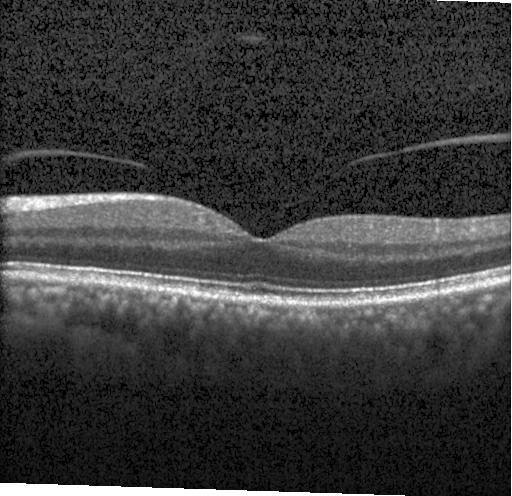
Retinal OCT cross-section, spectral-domain OCT, Heidelberg Spectralis, macular scan
Macular OCT: no CNV, DME, or drusen.